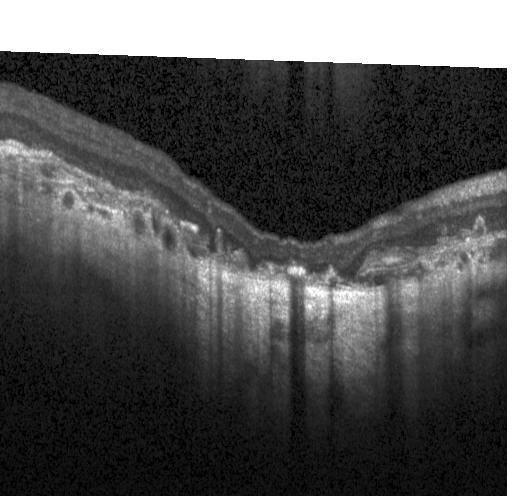 Retinal OCT B-scan — Choroidal neovascularization (CNV).